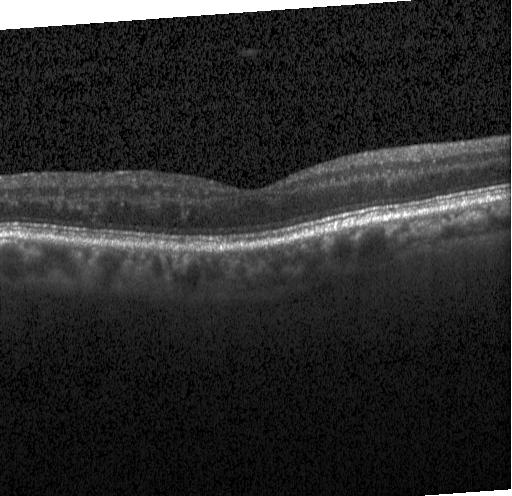

Retinal OCT cross-section. Finding: no choroidal neovascularization, no diabetic macular edema, and no drusen.